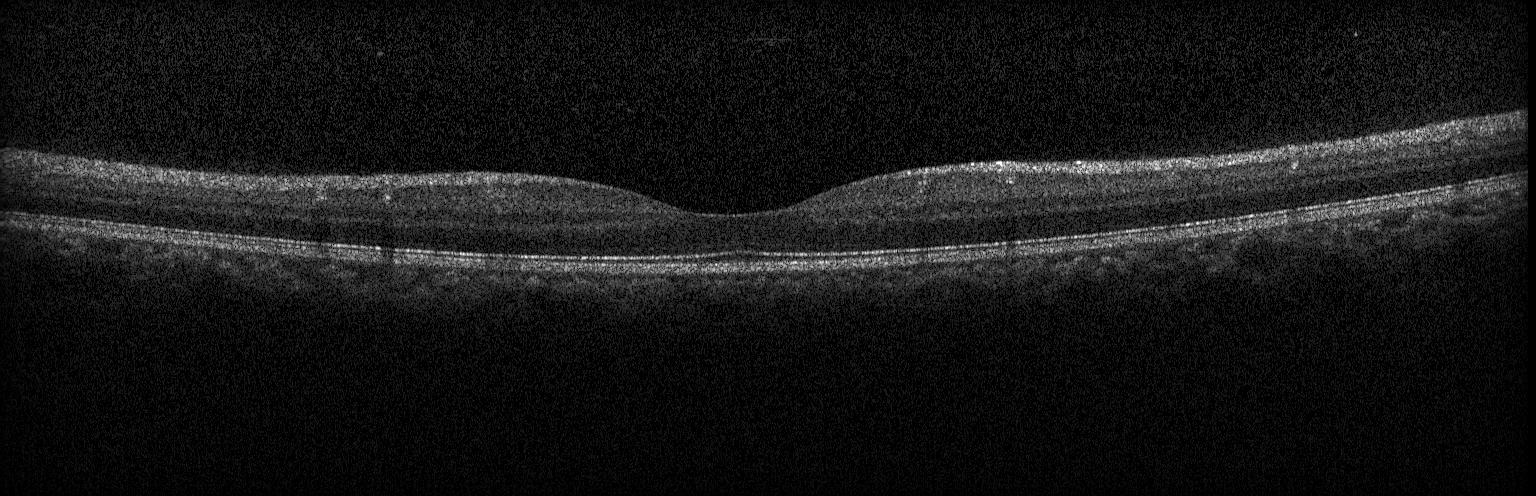
Through the macula. Spectral-domain optical coherence tomography. Retinal OCT cross-section.
Macular OCT: no choroidal neovascularization, diabetic macular edema, or drusen.